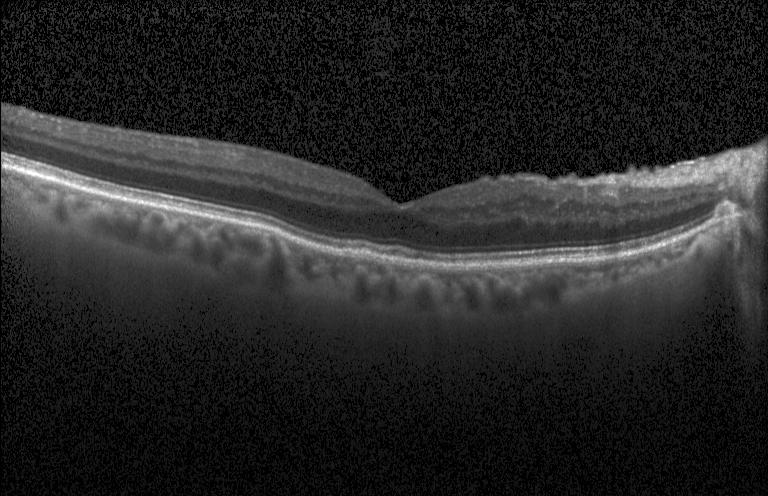
Retinal OCT B-scan
The scan shows no evidence of choroidal neovascularization, diabetic macular edema, or drusen.